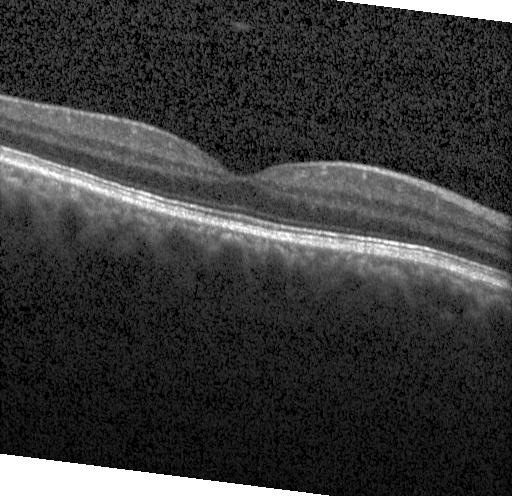 Finding: neither choroidal neovascularization, diabetic macular edema, nor drusen.